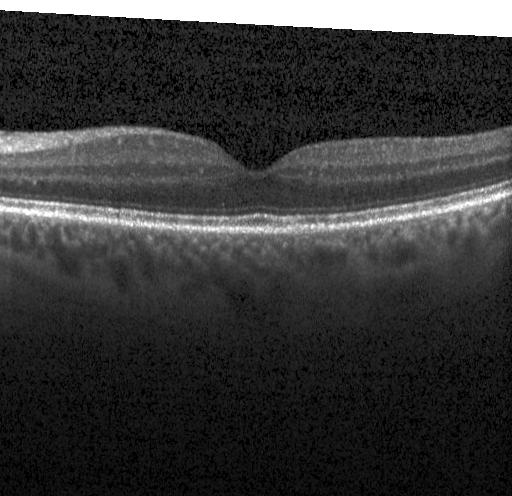 Spectral-domain OCT, optical coherence tomography B-scan, acquired on a Heidelberg Spectralis, centered on the fovea.
Macular OCT: no evidence of choroidal neovascularization, diabetic macular edema, or drusen.